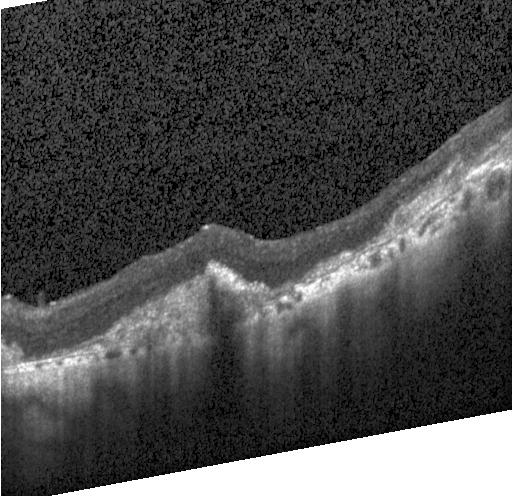

Diagnosis: a choroidal neovascular membrane.